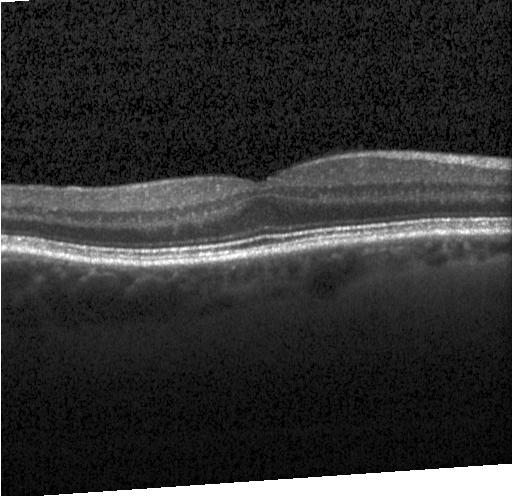 This B-scan demonstrates no evidence of choroidal neovascularization, diabetic macular edema, or drusen.